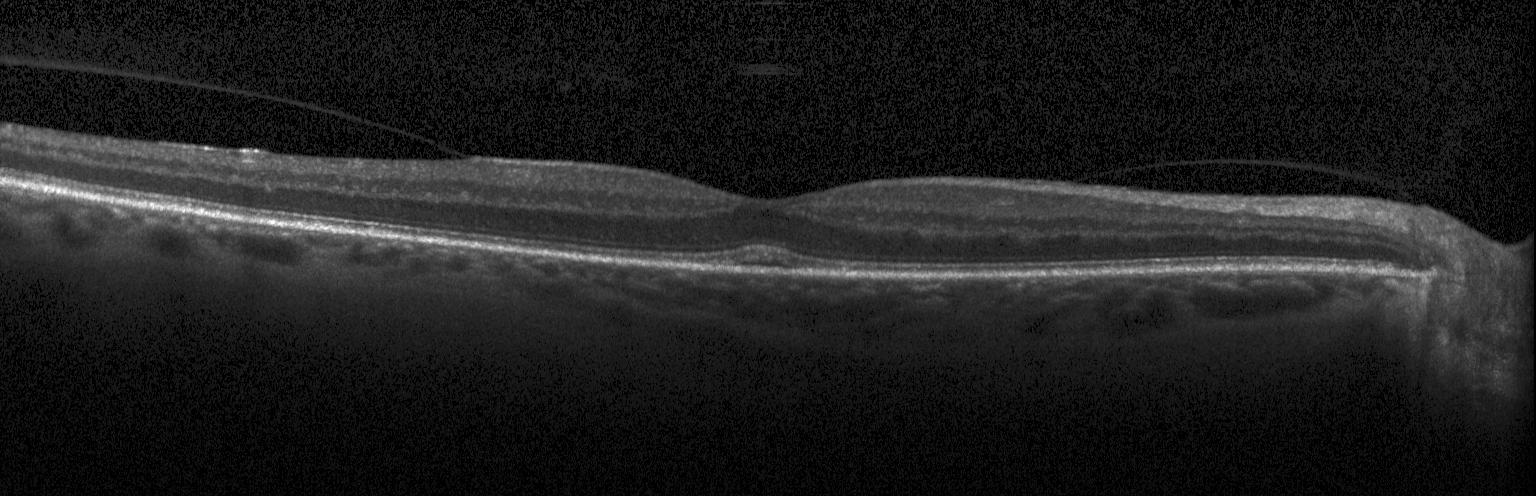 No choroidal neovascularization, no diabetic macular edema, and no drusen.